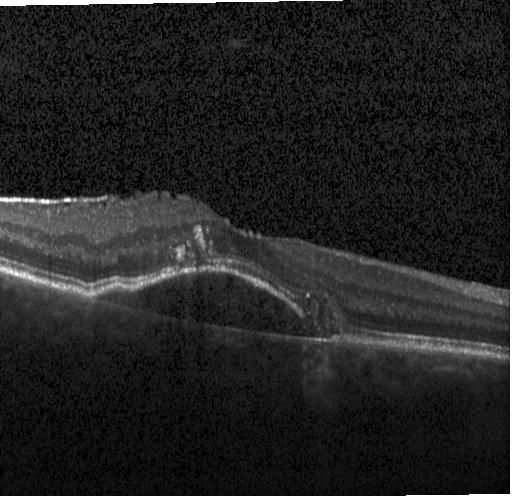

Retinal OCT cross-section · instrument: Heidelberg Spectralis
Diagnosis: CNV.